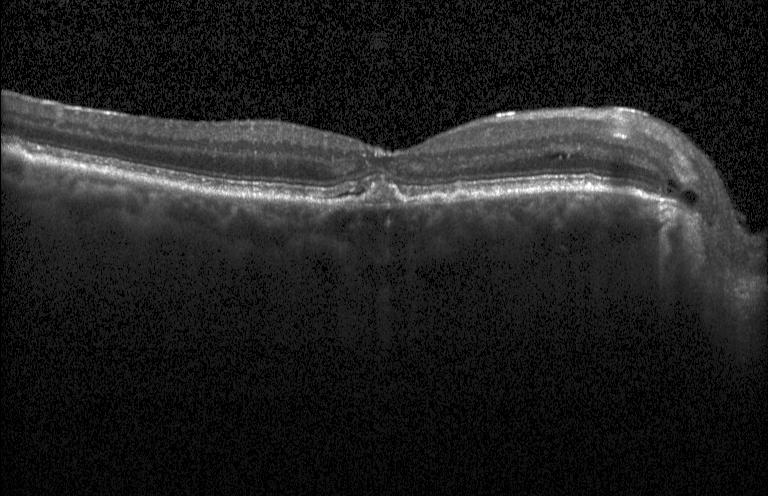

OCT line scan; horizontal scan through the fovea; spectral-domain OCT.
Impression: a choroidal neovascular membrane.